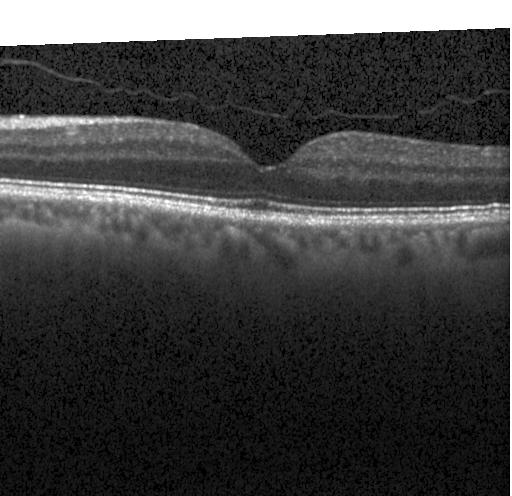 OCT B-scan showing no choroidal neovascularization, no diabetic macular edema, and no drusen.